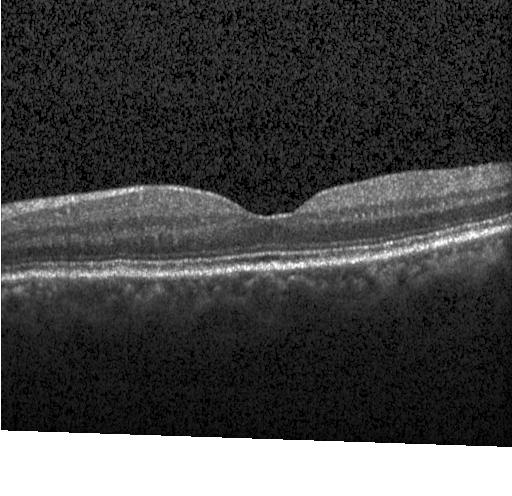
Horizontal scan through the fovea; instrument: Heidelberg Spectralis; optical coherence tomography B-scan — Impression: no choroidal neovascularization, no diabetic macular edema, and no drusen.